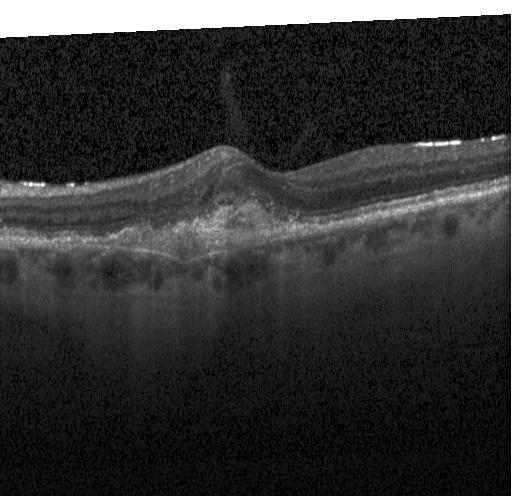

Retinal OCT B-scan · SD-OCT · fovea-centered.
Assessment: choroidal neovascularization (CNV).